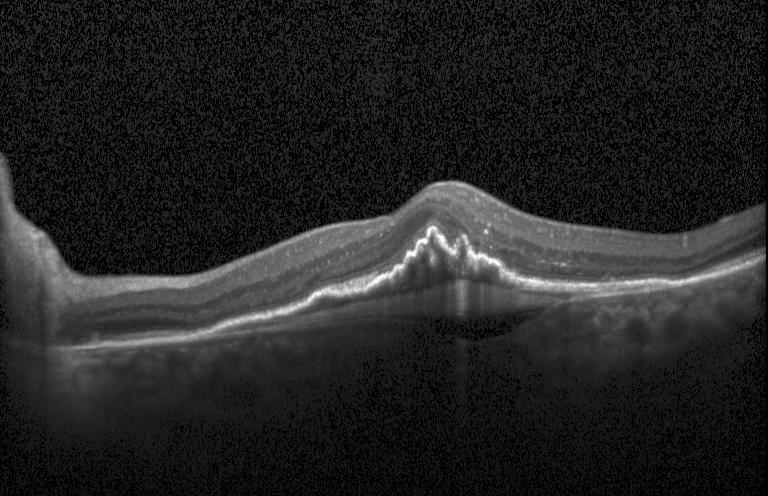
Retinal OCT cross-section showing choroidal neovascularization (CNV).